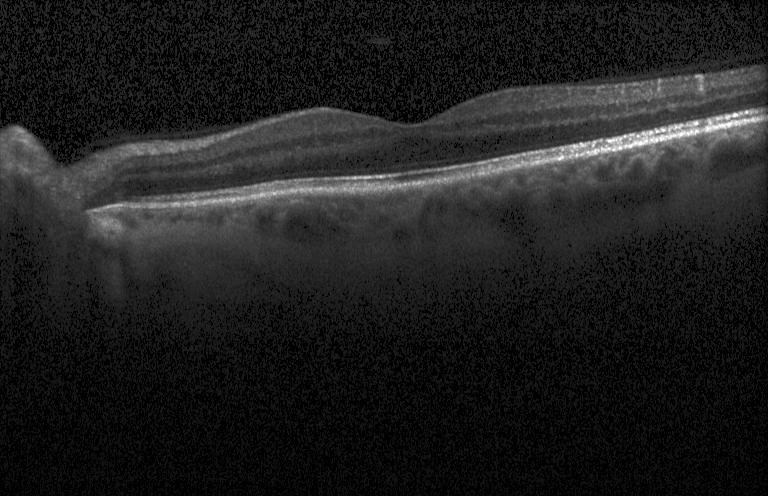 Diagnosis: neither CNV, DME, nor drusen.